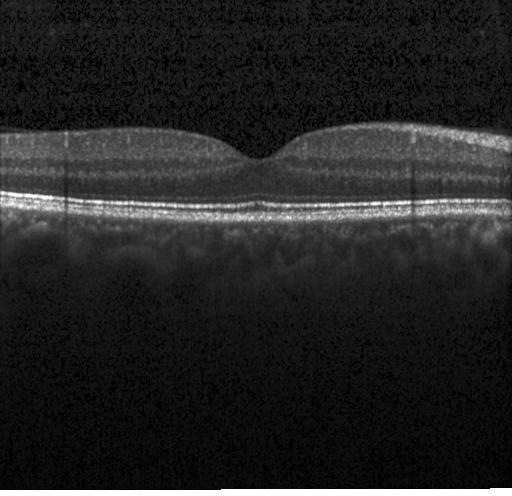
Retinal OCT B-scan — This B-scan demonstrates no choroidal neovascularization, no diabetic macular edema, and no drusen.